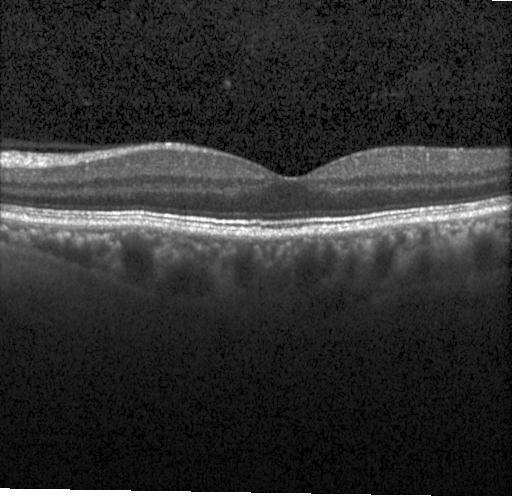 Spectral-domain optical coherence tomography; OCT line scan; Heidelberg Spectralis OCT system — No evidence of CNV, DME, or drusen.